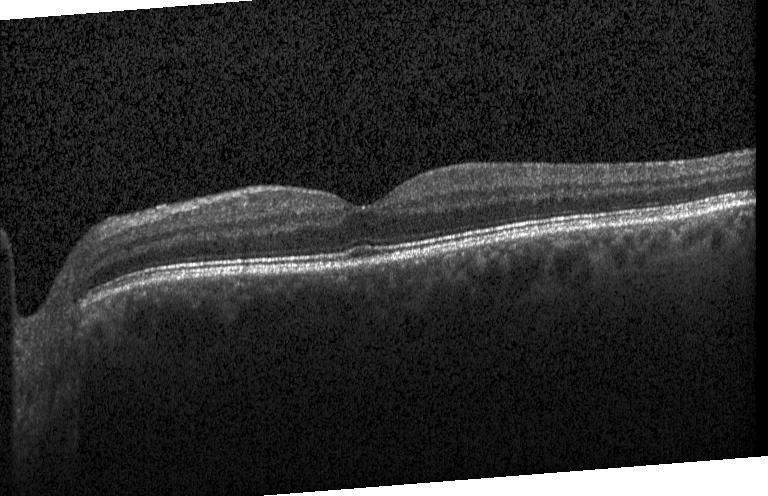

Horizontal scan through the fovea. Optical coherence tomography scan. Instrument: Heidelberg Spectralis
This B-scan demonstrates no choroidal neovascularization, no diabetic macular edema, and no drusen.